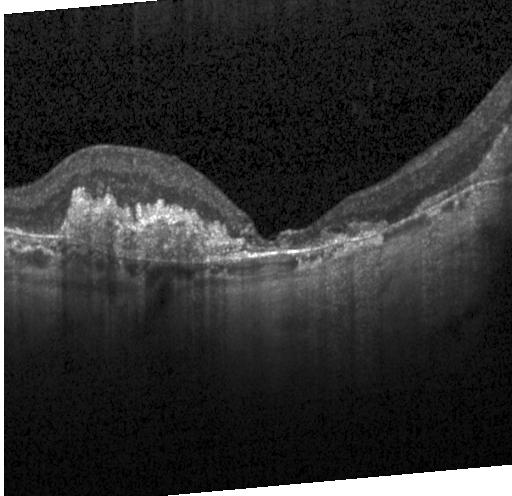 Optical coherence tomography B-scan; instrument: Heidelberg Spectralis; spectral-domain optical coherence tomography; fovea-centered. Assessment: a choroidal neovascular membrane.